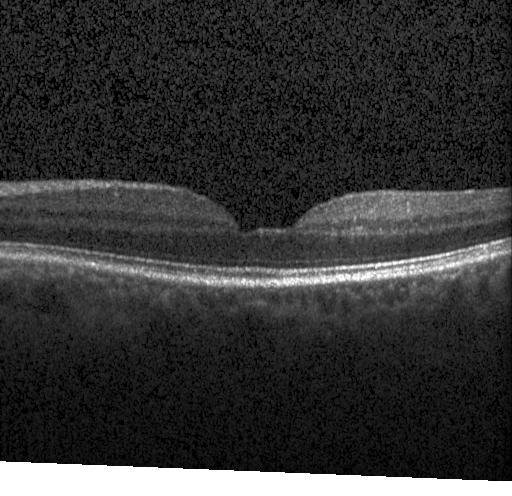

Spectral-domain OCT; OCT line scan — No choroidal neovascularization, diabetic macular edema, or drusen.